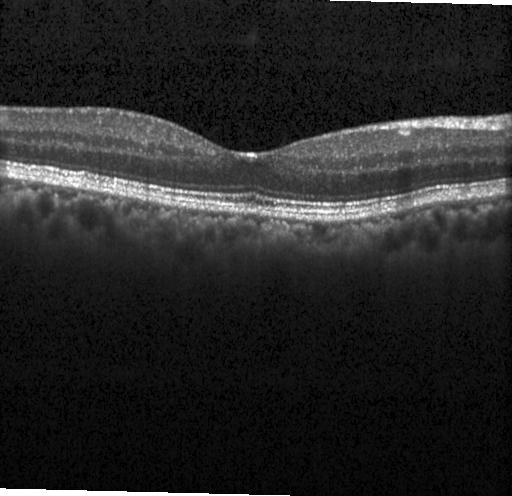 Retinal OCT B-scan; through the macula
The scan shows no choroidal neovascularization, diabetic macular edema, or drusen.